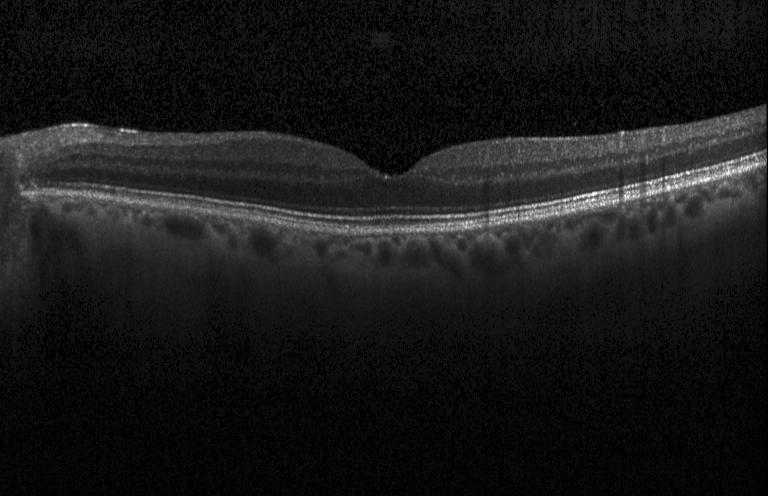
Spectral-domain OCT. Retinal OCT B-scan. Through the macula. Heidelberg Spectralis OCT system — Finding: no choroidal neovascularization, diabetic macular edema, or drusen.